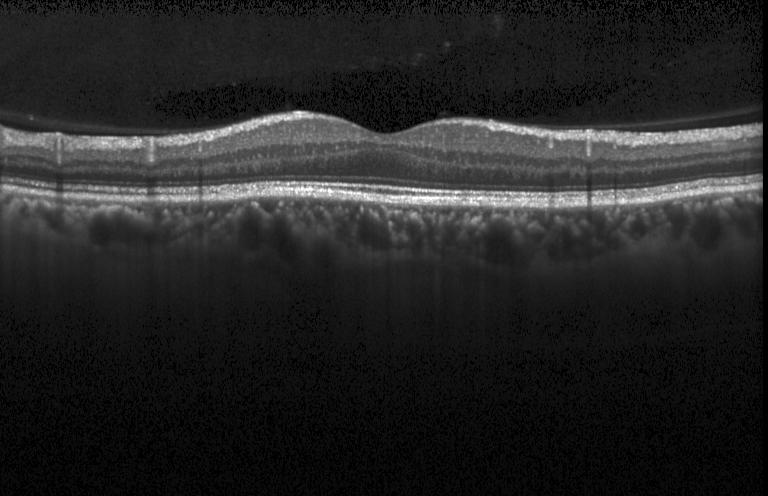
Optical coherence tomography scan · instrument: Heidelberg Spectralis — Diagnosis: neither CNV, DME, nor drusen.